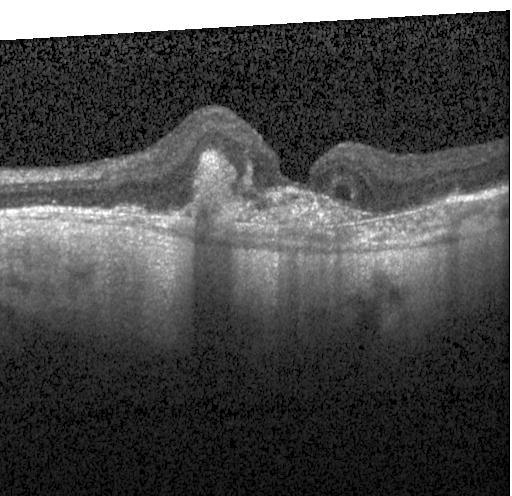
Heidelberg Spectralis OCT system · optical coherence tomography B-scan · SD-OCT · centered on the fovea.
This B-scan demonstrates a choroidal neovascular membrane.